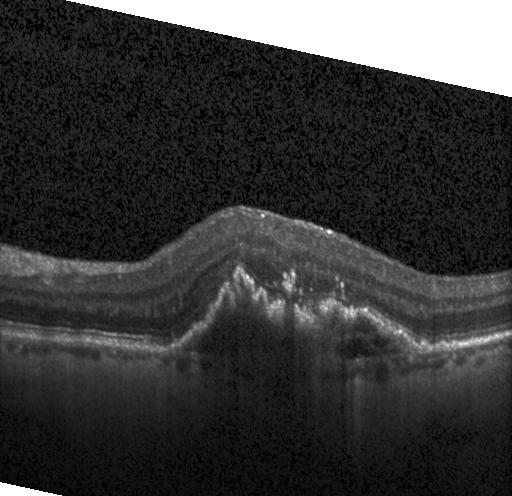

Fovea-centered · Heidelberg Spectralis OCT system · OCT line scan · spectral-domain OCT. Diagnosis: a choroidal neovascular membrane.